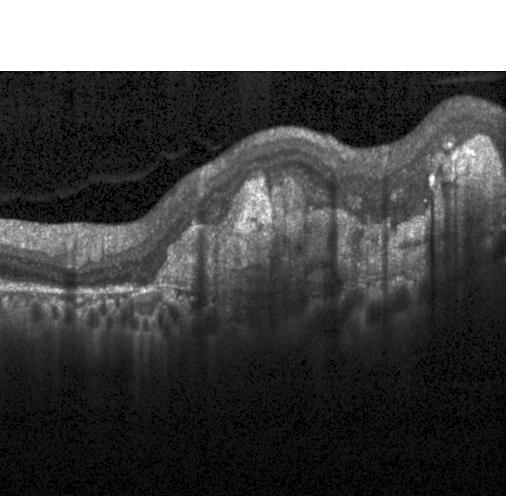
Retinal OCT cross-section, spectral-domain OCT. Assessment: a choroidal neovascular membrane.